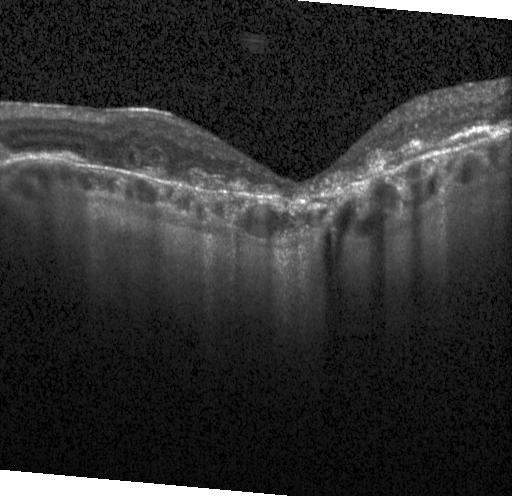

Fovea-centered · Heidelberg Spectralis OCT system · retinal OCT B-scan · SD-OCT.
A choroidal neovascular membrane.